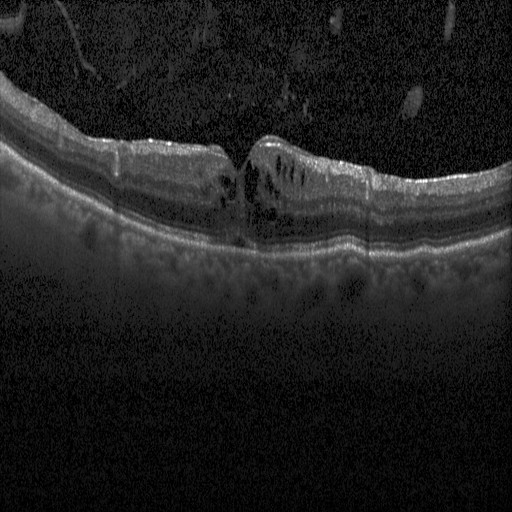
Retinal OCT cross-section, spectral-domain OCT
Diagnosis: diabetic macular edema.